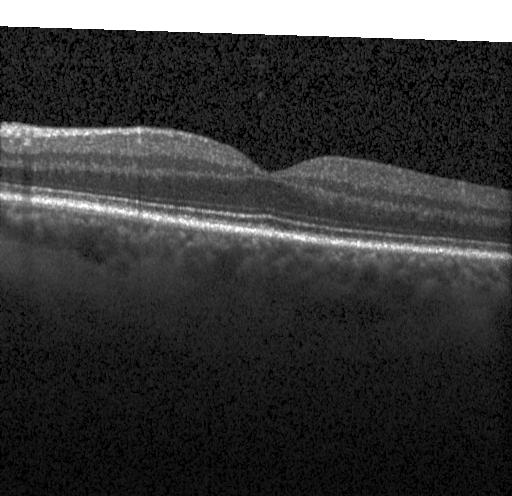 Instrument: Heidelberg Spectralis · spectral-domain optical coherence tomography · optical coherence tomography scan — Diagnosis: no CNV, DME, or drusen.